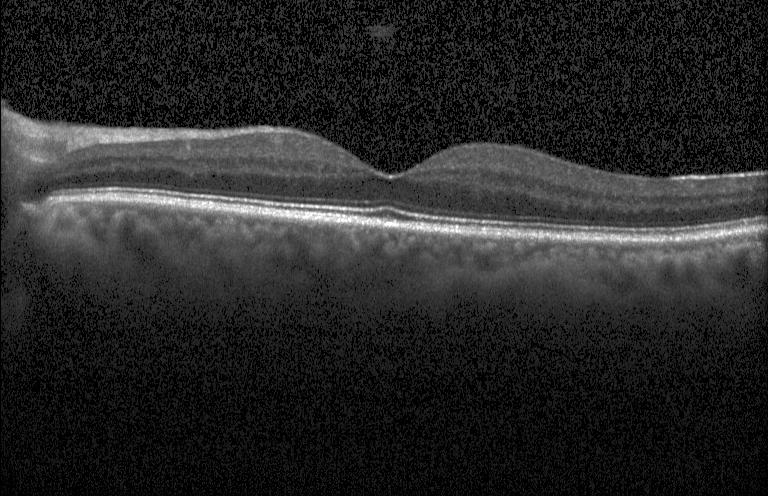 Diagnosis: no choroidal neovascularization, no diabetic macular edema, and no drusen.